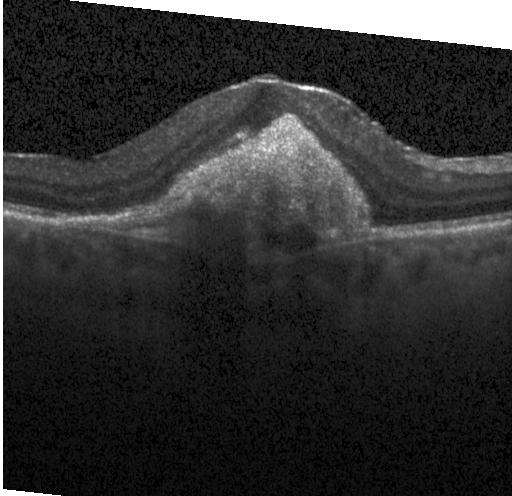

Optical coherence tomography B-scan; Heidelberg Spectralis; fovea-centered
Finding: a choroidal neovascular membrane.